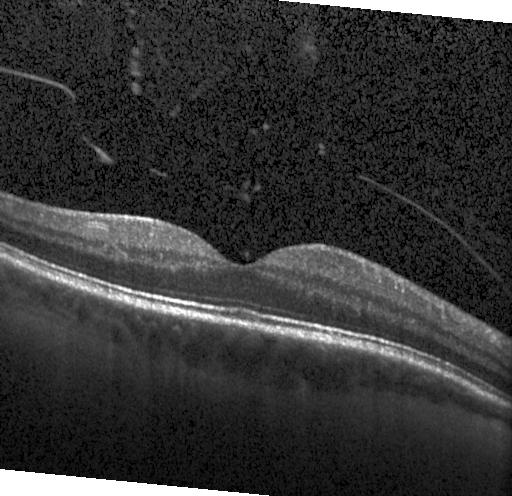
OCT B-scan; SD-OCT; fovea-centered.
OCT finding: no evidence of choroidal neovascularization, diabetic macular edema, or drusen.